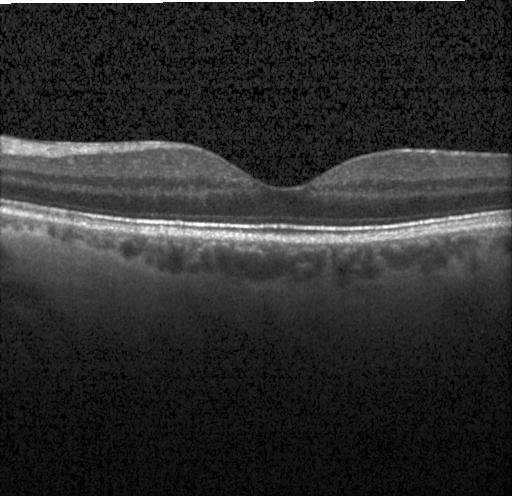
Acquired on a Heidelberg Spectralis · through the macula · spectral-domain optical coherence tomography · optical coherence tomography scan. Diagnosis: neither CNV, DME, nor drusen.